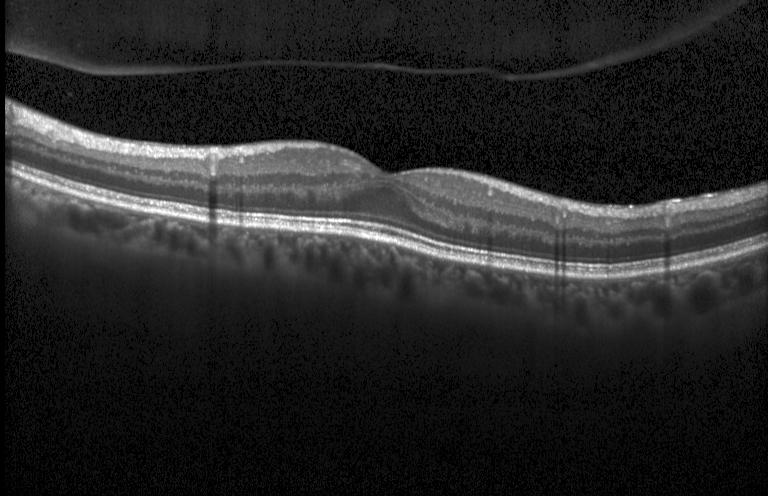
The scan shows no evidence of CNV, DME, or drusen.